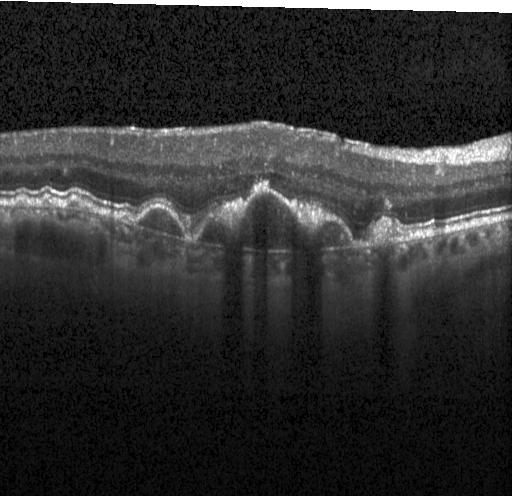
OCT line scan; spectral-domain OCT; instrument: Heidelberg Spectralis. Finding: CNV.